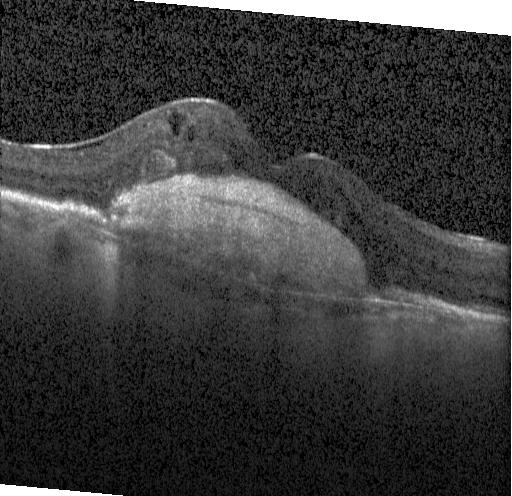
Retinal OCT B-scan, spectral-domain optical coherence tomography, instrument: Heidelberg Spectralis, macular scan. Macular OCT: choroidal neovascularization (CNV).